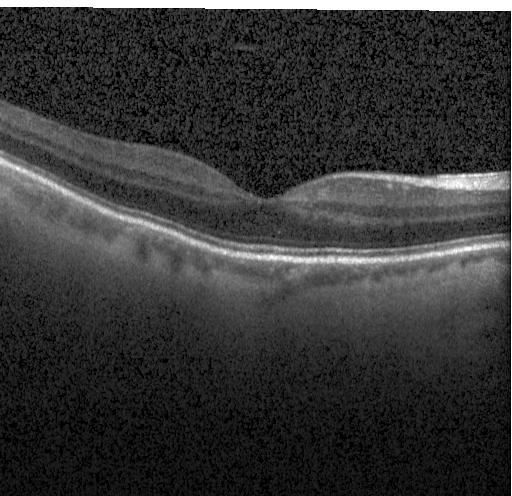 Retinal OCT B-scan · through the macula — The scan shows no CNV, DME, or drusen.